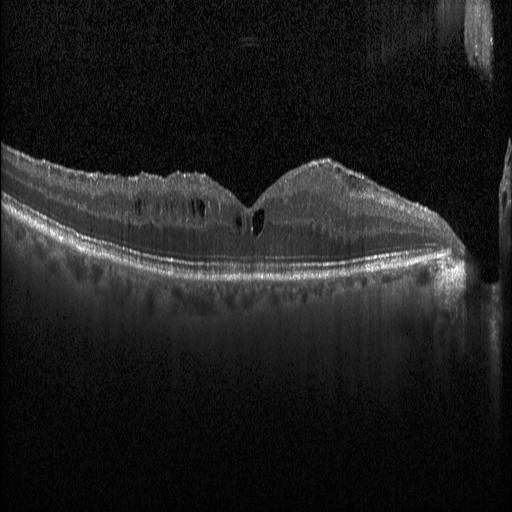

OCT B-scan, spectral-domain OCT, centered on the fovea, Heidelberg Spectralis
Finding: diabetic macular edema.